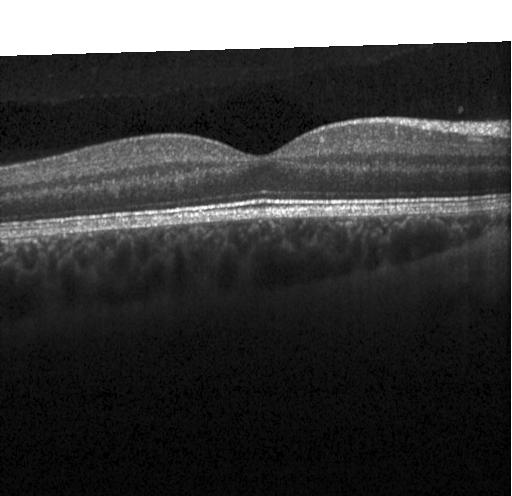

Acquired on a Heidelberg Spectralis; SD-OCT; through the macula; optical coherence tomography B-scan — Diagnosis: no CNV, no DME, and no drusen.